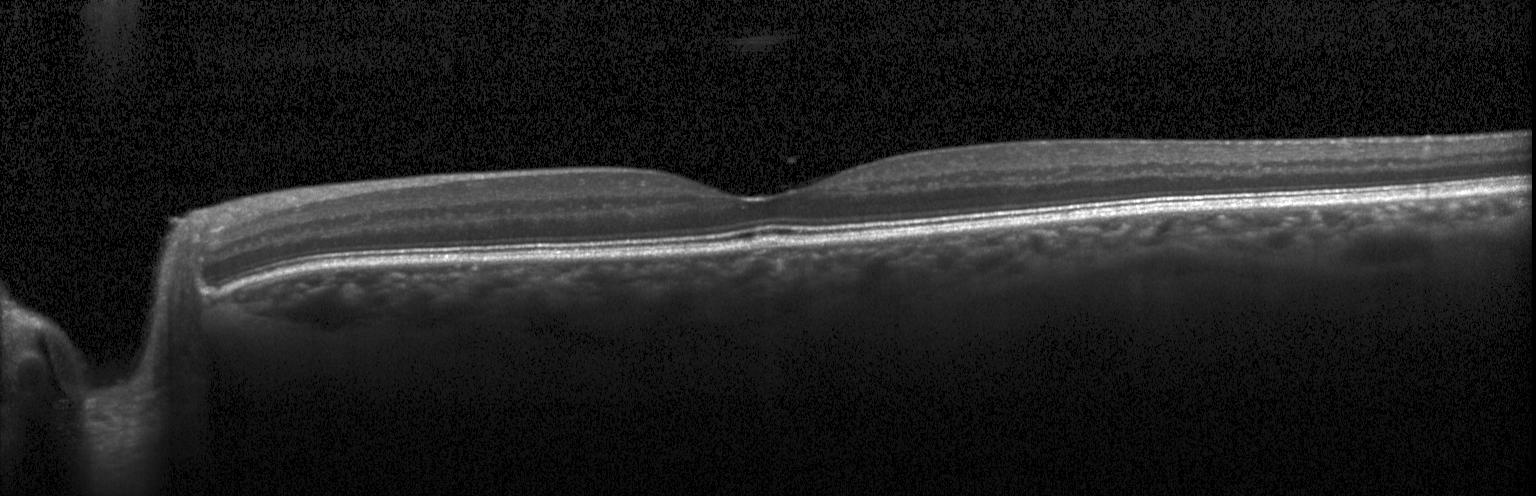 Spectral-domain OCT · optical coherence tomography scan. Dx: no CNV, no DME, and no drusen.